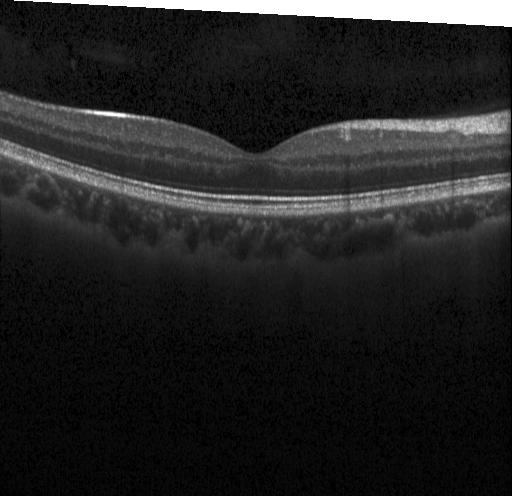
Through the macula; Heidelberg Spectralis; retinal OCT B-scan.
Assessment: no evidence of choroidal neovascularization, diabetic macular edema, or drusen.